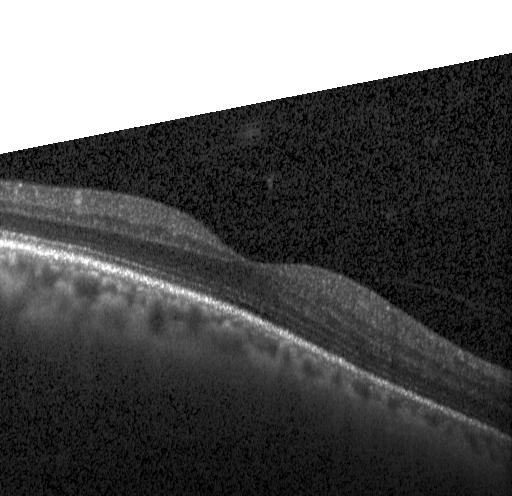

OCT finding: no choroidal neovascularization, no diabetic macular edema, and no drusen.